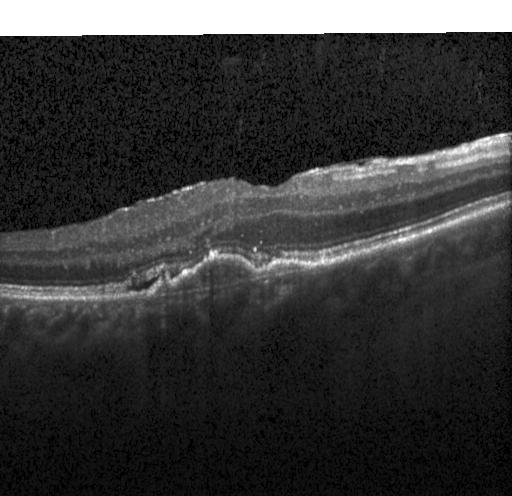
Through the macula · OCT line scan — Finding: a choroidal neovascular membrane.